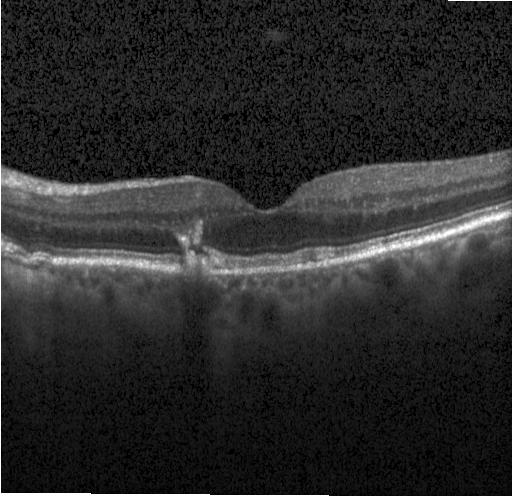 Finding: drusen.